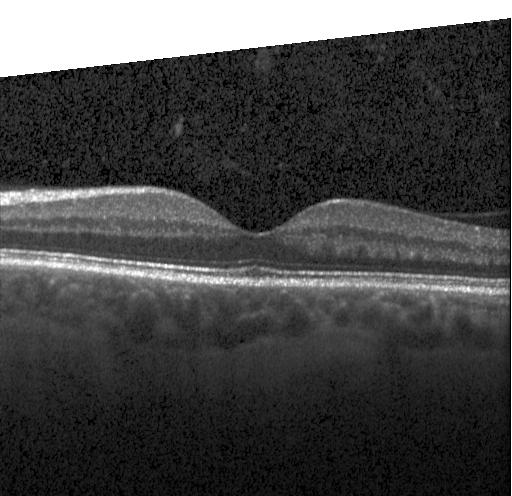
Spectral-domain optical coherence tomography · optical coherence tomography scan.
Dx: neither CNV, DME, nor drusen.